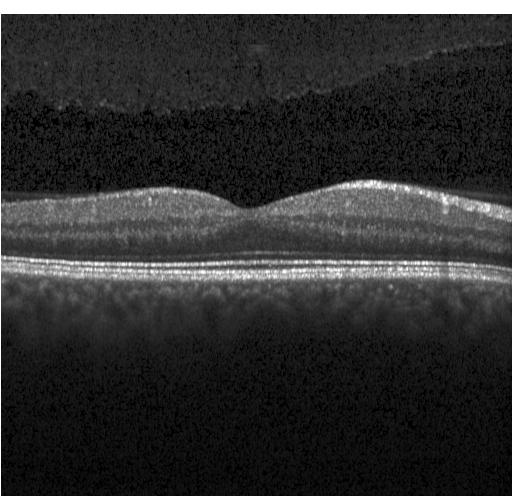

Optical coherence tomography scan.
This B-scan demonstrates no CNV, DME, or drusen.